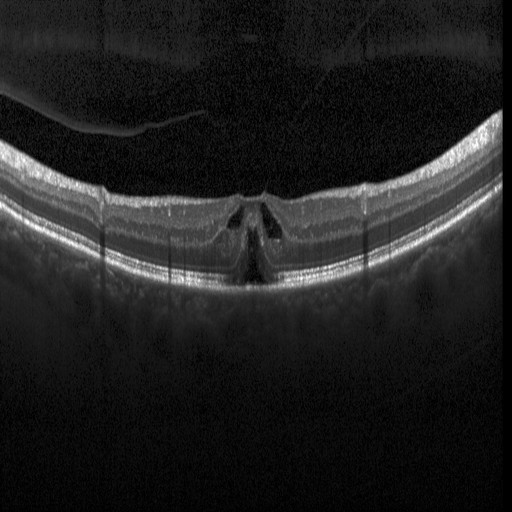
OCT B-scan. Fovea-centered.
Diagnosis: diabetic macular edema (DME).